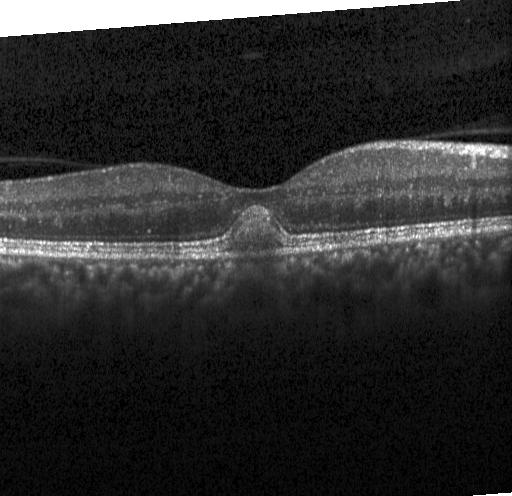
SD-OCT, retinal OCT cross-section, instrument: Heidelberg Spectralis — Diagnosis: choroidal neovascularization.